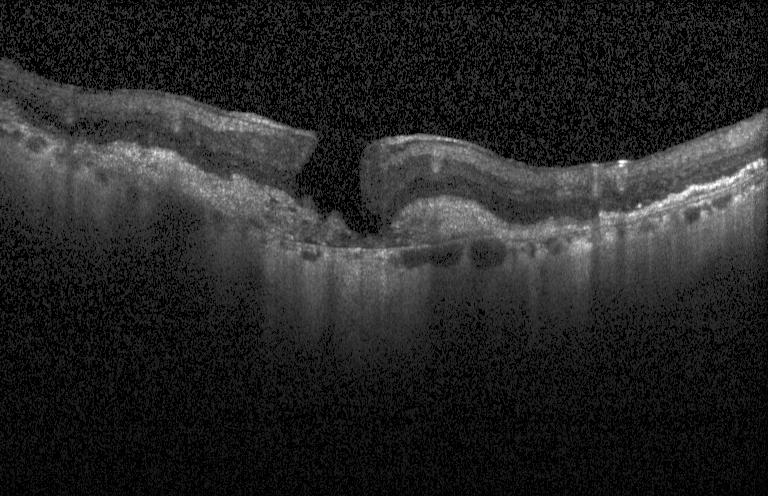

Macular OCT demonstrating choroidal neovascularization (CNV).